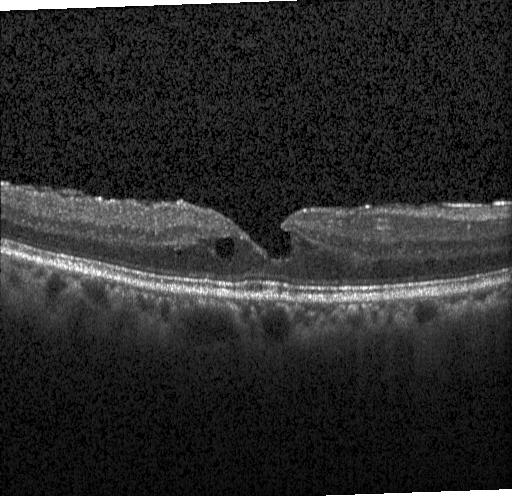

Diagnosis: DME.